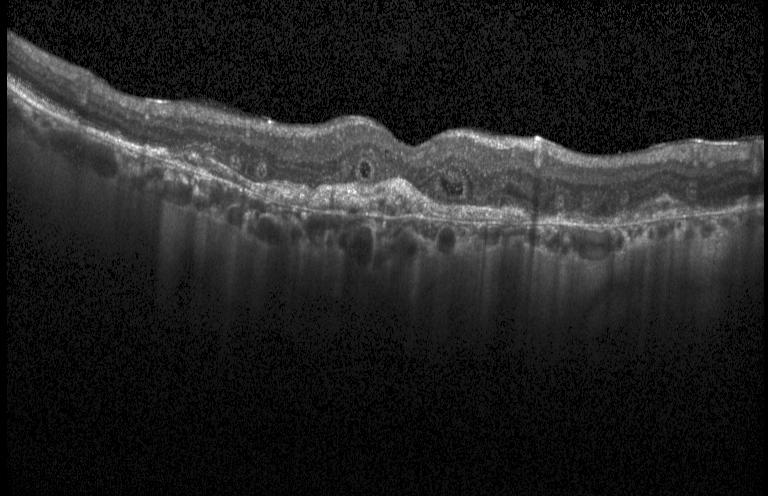
Finding: a choroidal neovascular membrane.